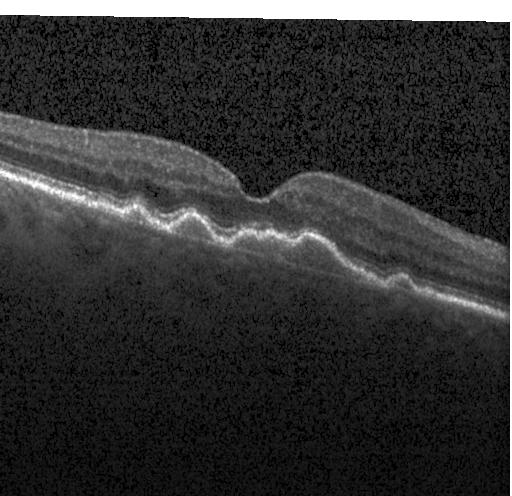
Optical coherence tomography scan.
Dx: CNV.